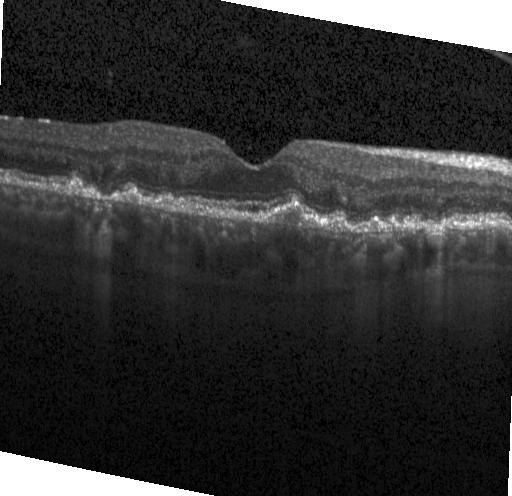
Spectral-domain optical coherence tomography. OCT B-scan. Dx: sub-RPE drusenoid deposits.